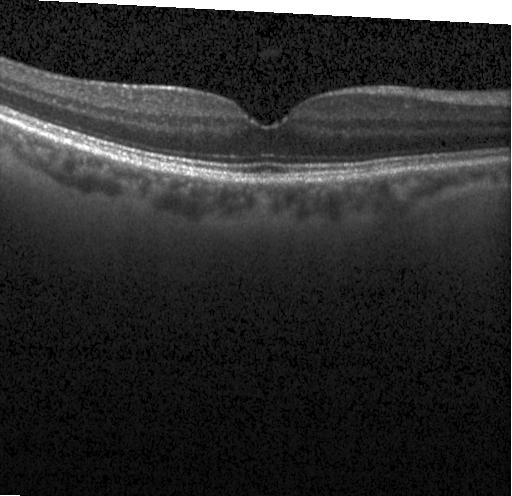

Retinal OCT B-scan. This B-scan demonstrates no evidence of CNV, DME, or drusen.